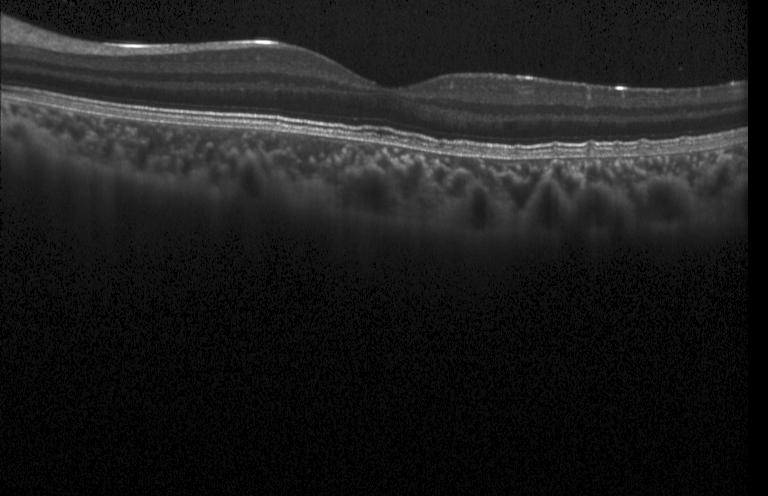

Retinal OCT B-scan — The scan shows no evidence of CNV, DME, or drusen.